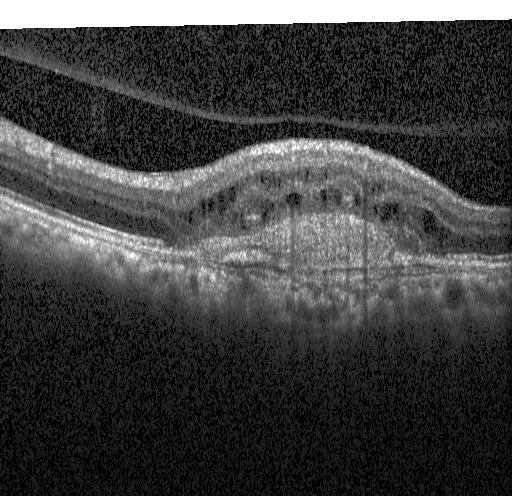
Macular OCT: a choroidal neovascular membrane.